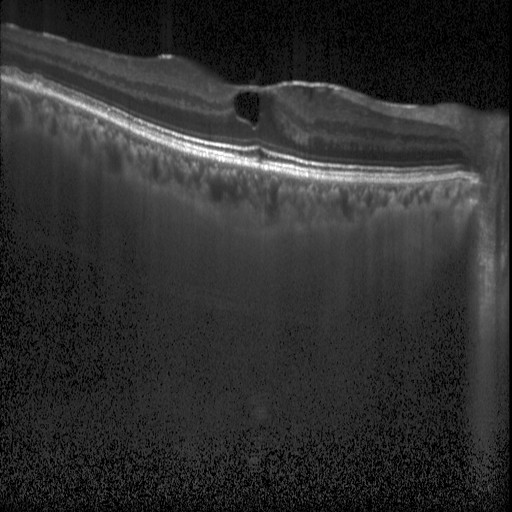
Retinal OCT B-scan · SD-OCT.
Finding: diabetic macular edema.